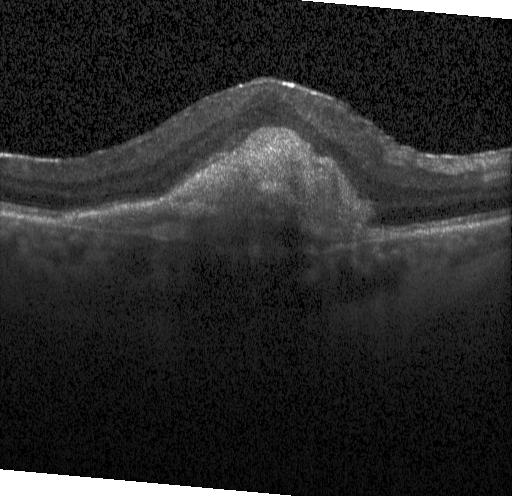
OCT line scan · macular scan · spectral-domain OCT — Choroidal neovascularization.